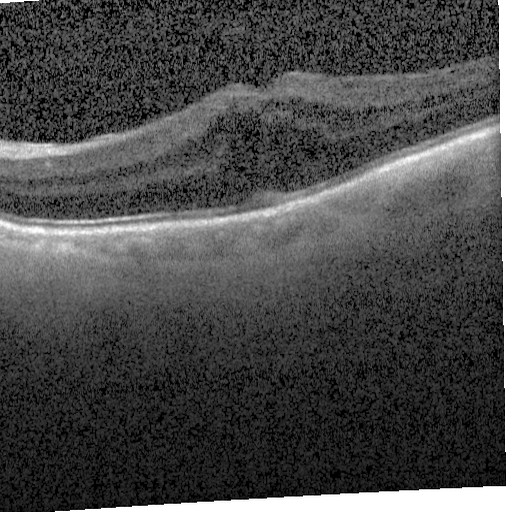 OCT line scan; spectral-domain optical coherence tomography; horizontal scan through the fovea. Finding: diabetic macular edema.